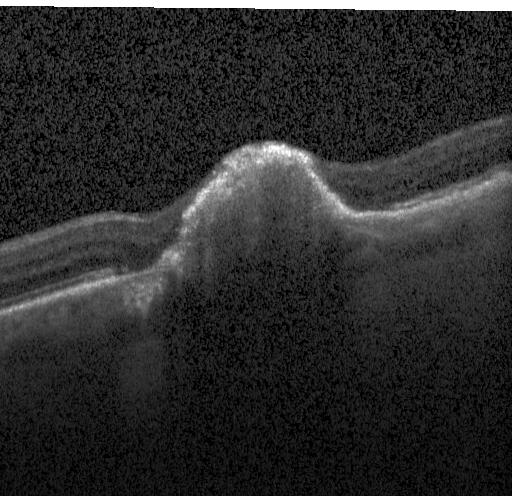

Finding: a choroidal neovascular membrane.